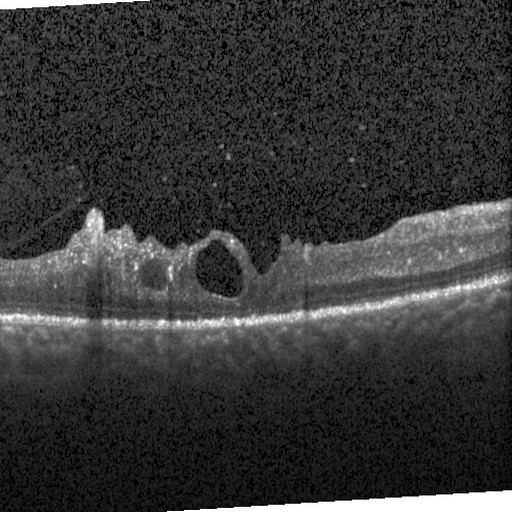
Heidelberg Spectralis. Fovea-centered. Optical coherence tomography scan. The scan shows diabetic macular edema (DME).